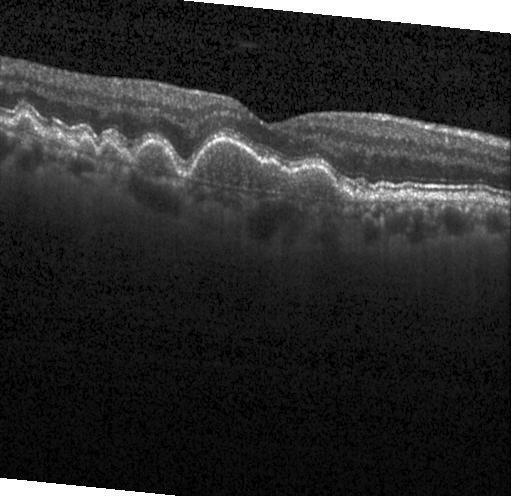
The scan shows sub-RPE drusenoid deposits.